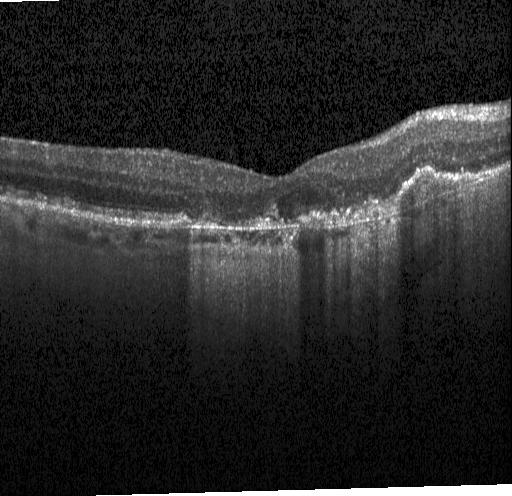 Heidelberg Spectralis; spectral-domain optical coherence tomography; OCT line scan; macular scan — Diagnosis: CNV.